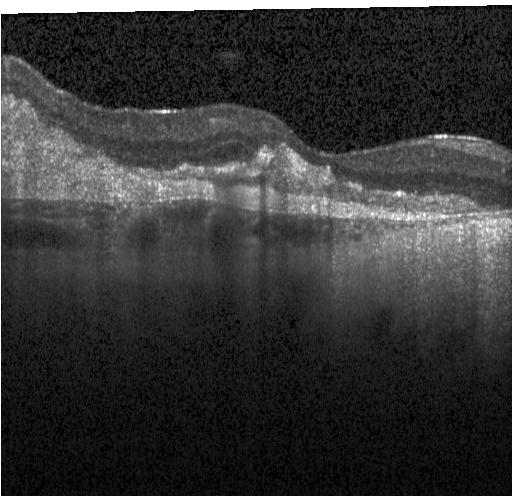
Spectral-domain OCT B-scan: choroidal neovascularization.